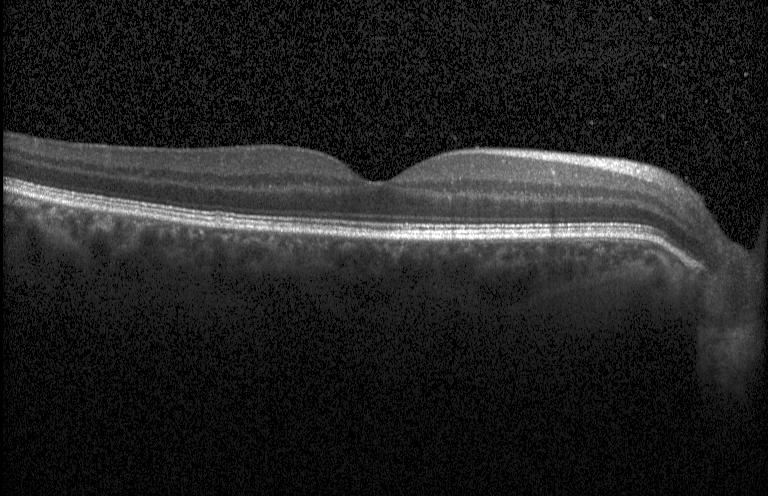

OCT B-scan; acquired on a Heidelberg Spectralis; spectral-domain optical coherence tomography.
Diagnosis: no choroidal neovascularization, diabetic macular edema, or drusen.